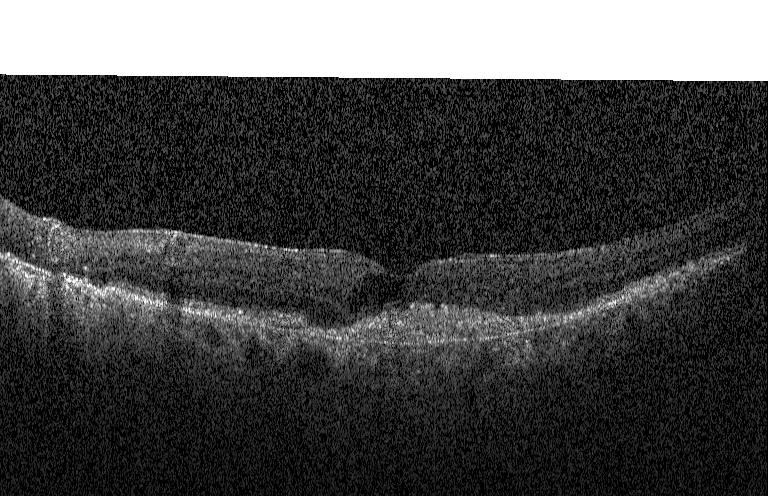 Dx: choroidal neovascularization (CNV).